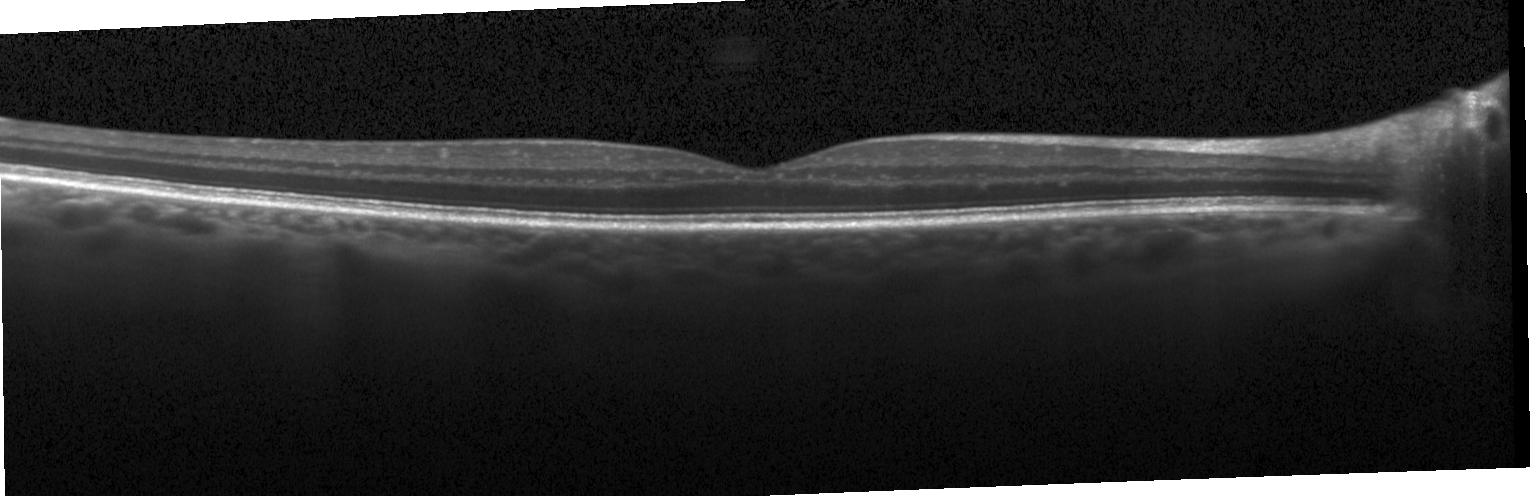 Diagnosis: no choroidal neovascularization, diabetic macular edema, or drusen.